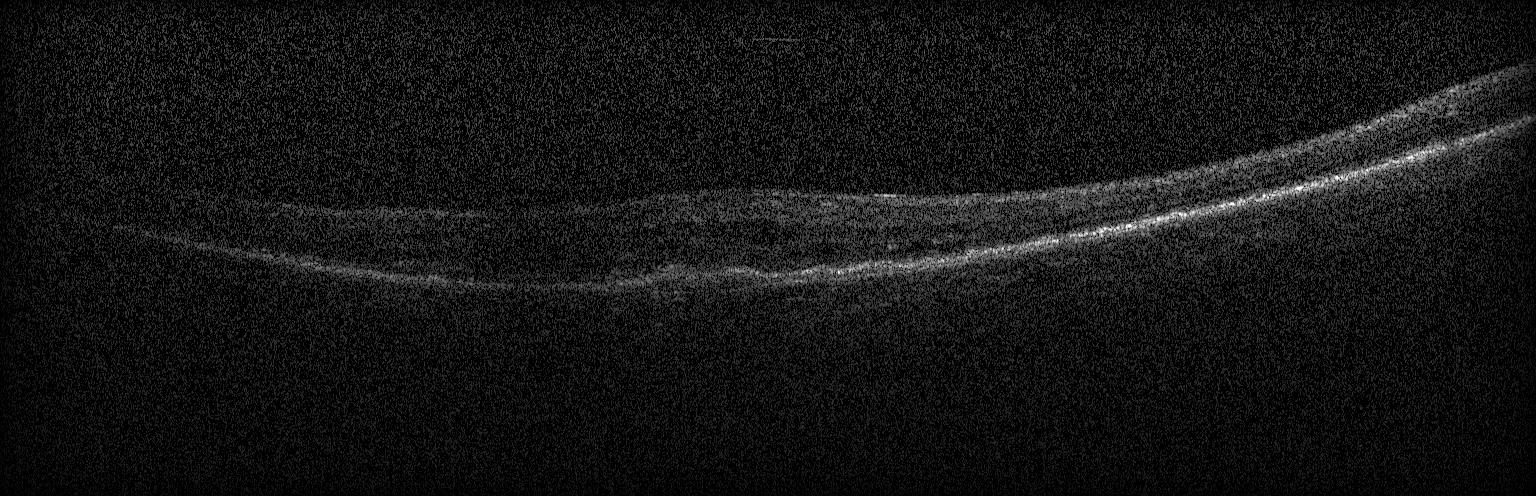
Impression: choroidal neovascularization.